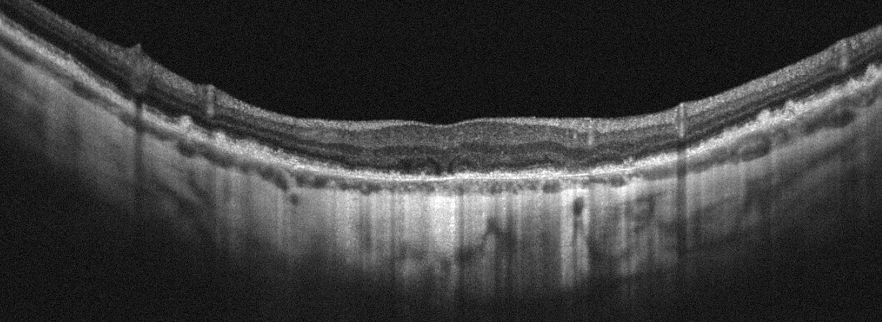
OCT line scan. Left eye. Impression: AMD.